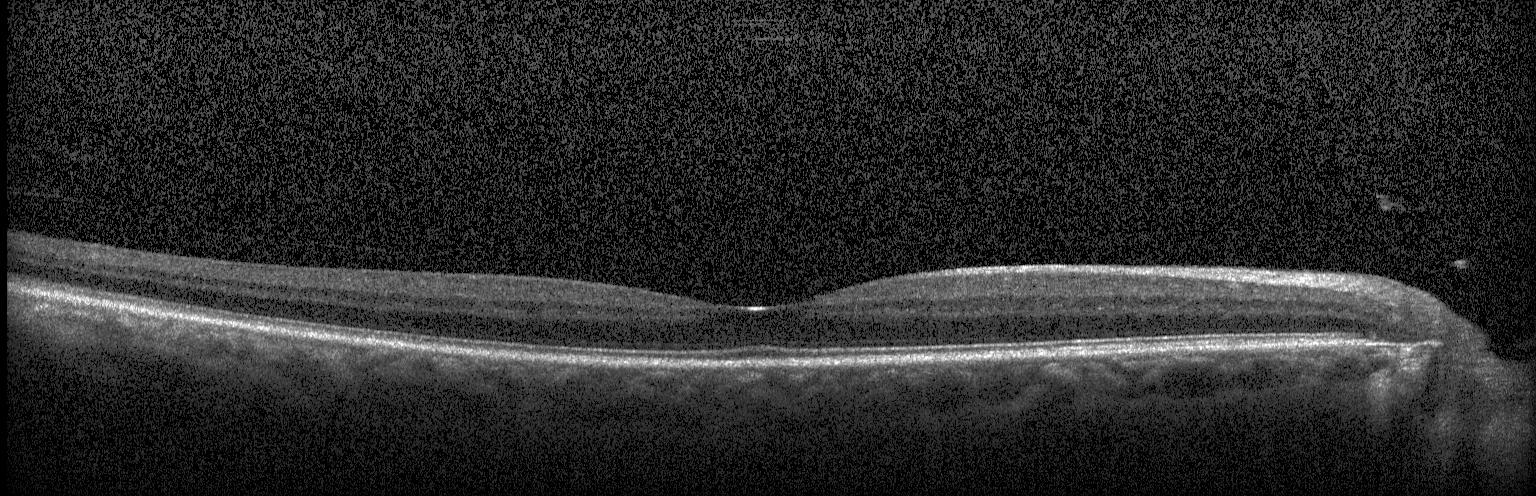 Horizontal scan through the fovea · OCT line scan · instrument: Heidelberg Spectralis — Neither CNV, DME, nor drusen.